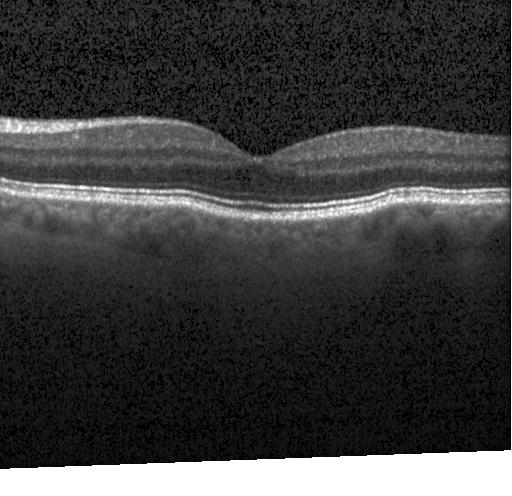
OCT line scan — Impression: neither choroidal neovascularization, diabetic macular edema, nor drusen.